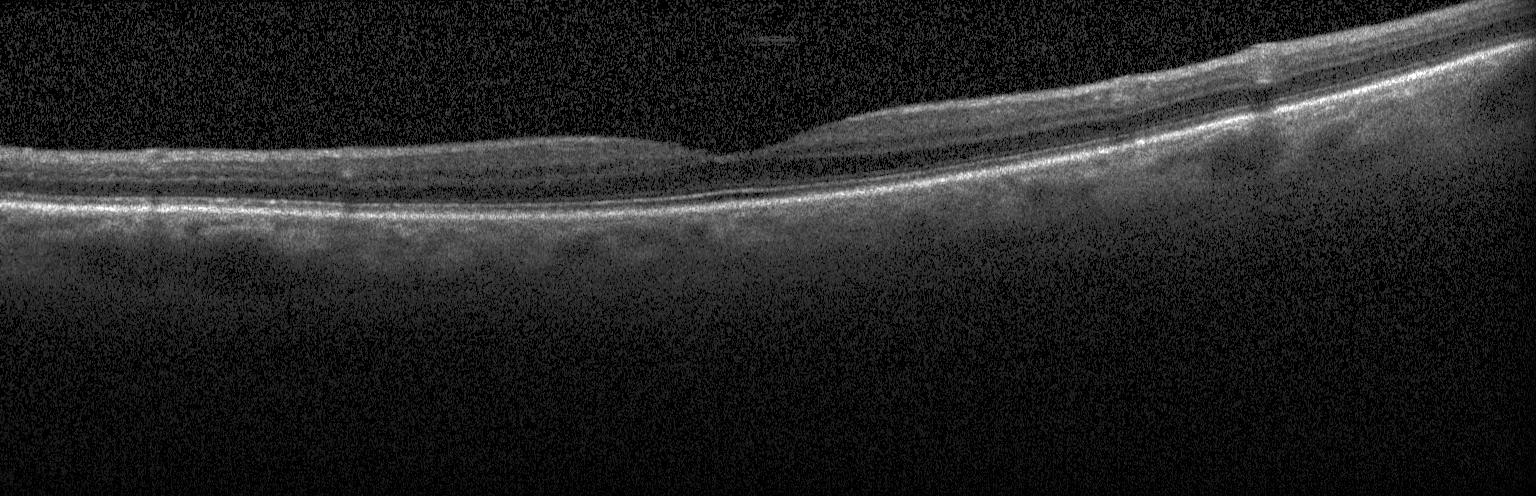 Spectral-domain OCT · optical coherence tomography B-scan. Finding: neither choroidal neovascularization, diabetic macular edema, nor drusen.